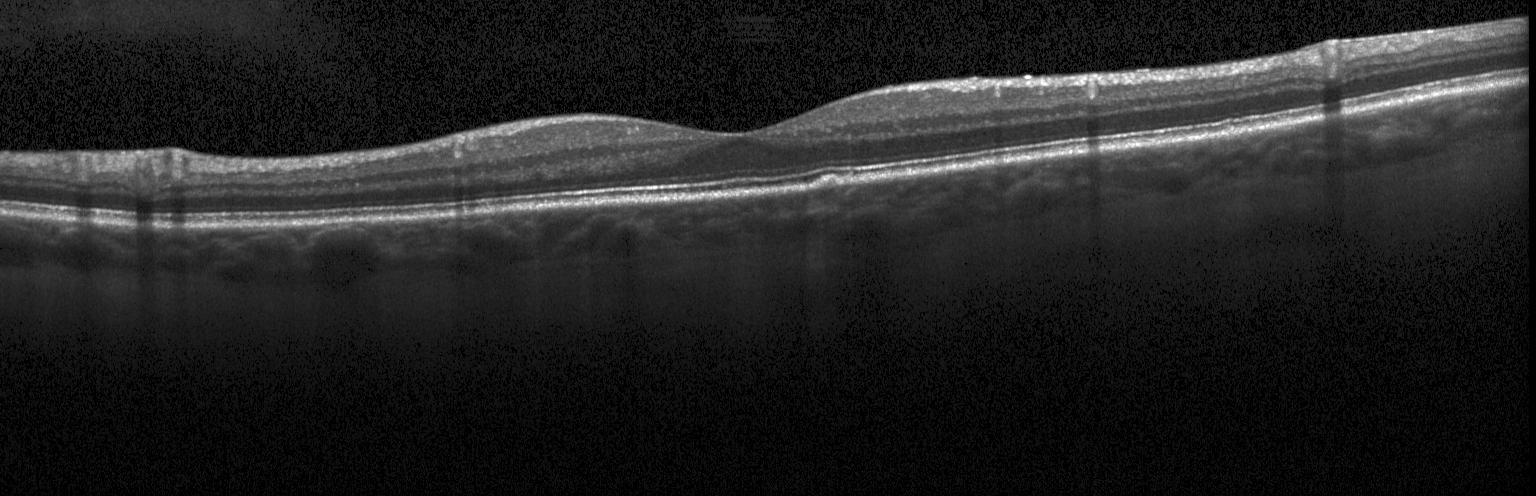 Macular scan, OCT line scan, spectral-domain OCT
The scan shows sub-RPE drusenoid deposits.